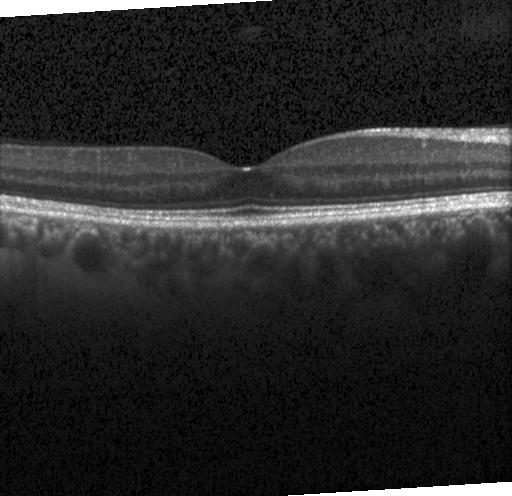
Retinal OCT B-scan. Macular OCT: neither choroidal neovascularization, diabetic macular edema, nor drusen.